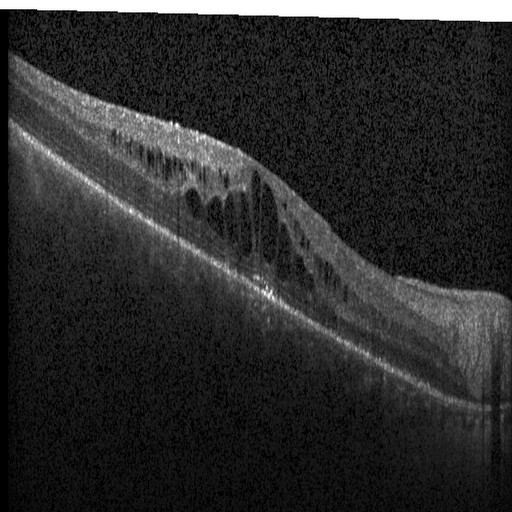

OCT line scan. Horizontal scan through the fovea. SD-OCT. The scan shows diabetic macular edema (DME).